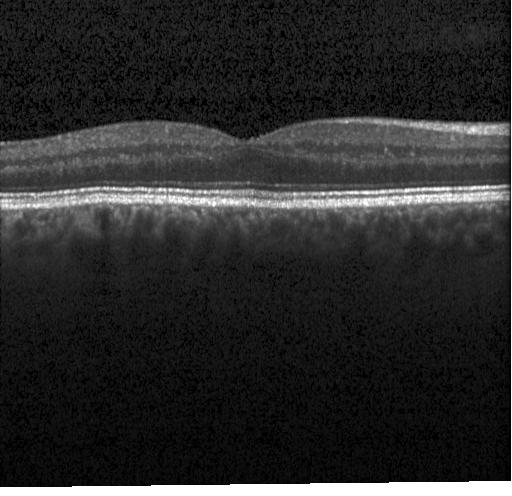
Retinal OCT cross-section. Impression: neither CNV, DME, nor drusen.